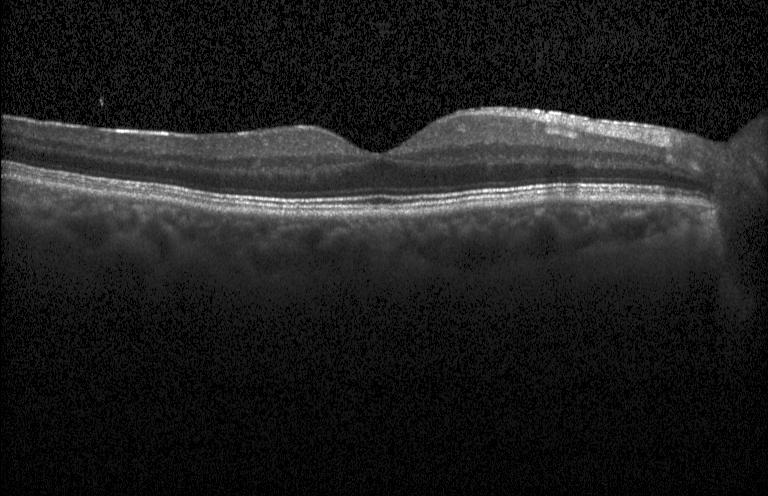 Assessment: no choroidal neovascularization, no diabetic macular edema, and no drusen.